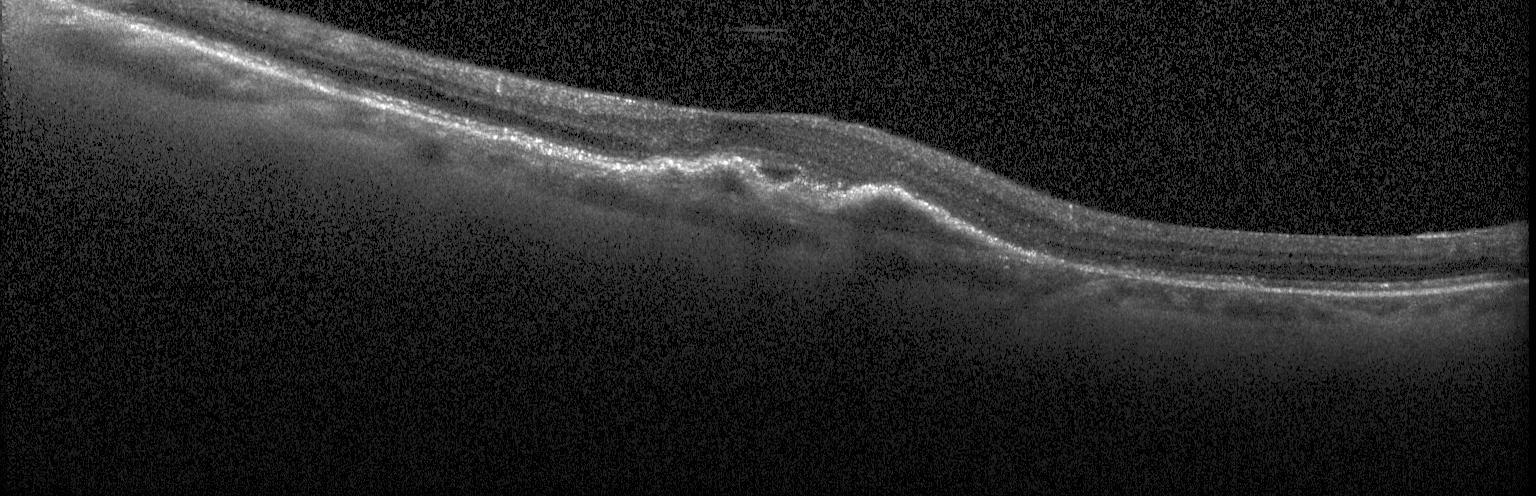

Spectral-domain OCT; OCT line scan; instrument: Heidelberg Spectralis; fovea-centered. The scan shows a choroidal neovascular membrane.